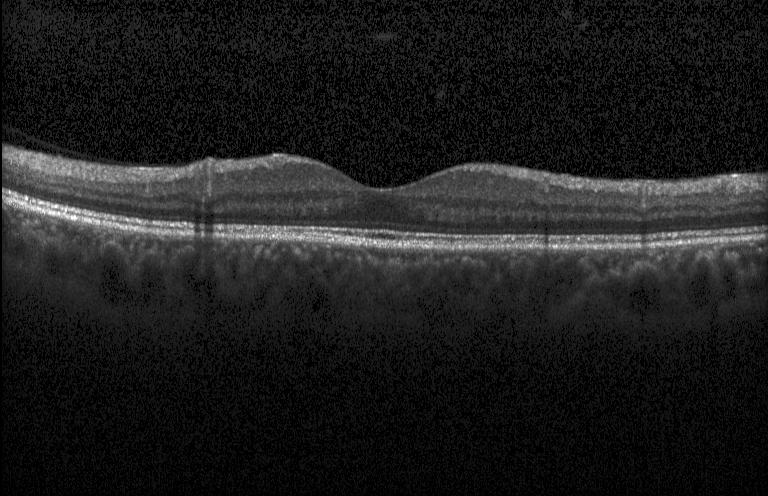 Impression: neither choroidal neovascularization, diabetic macular edema, nor drusen.